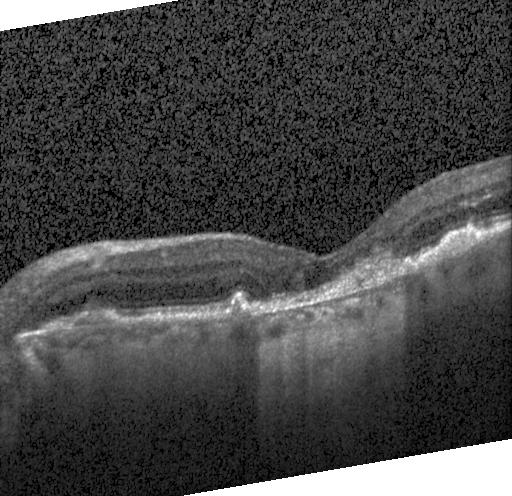
Macular scan. Spectral-domain optical coherence tomography. Retinal OCT B-scan — Diagnosis: CNV.